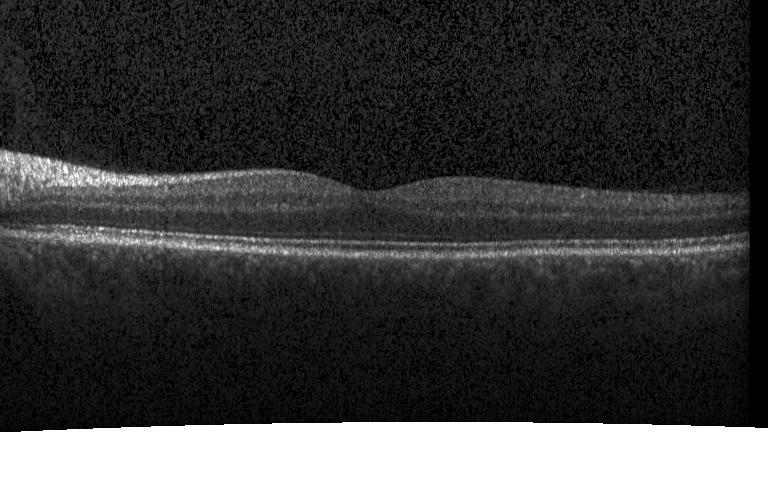
Optical coherence tomography B-scan.
No CNV, no DME, and no drusen.